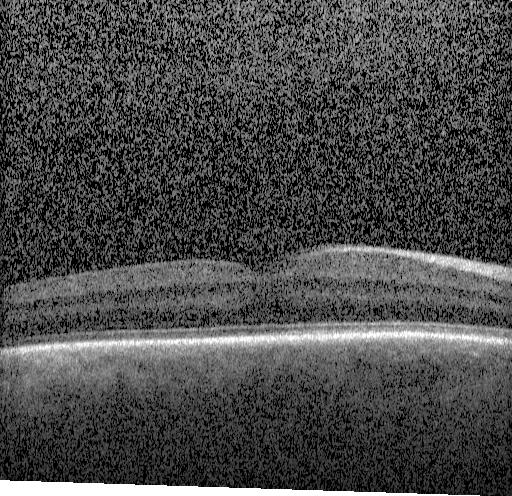
Finding: no choroidal neovascularization, no diabetic macular edema, and no drusen.